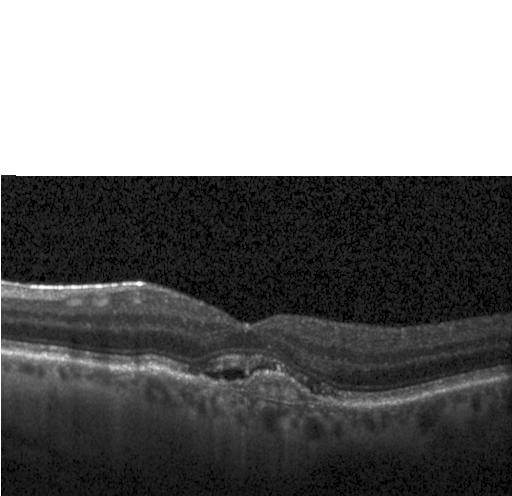 OCT finding: a choroidal neovascular membrane.